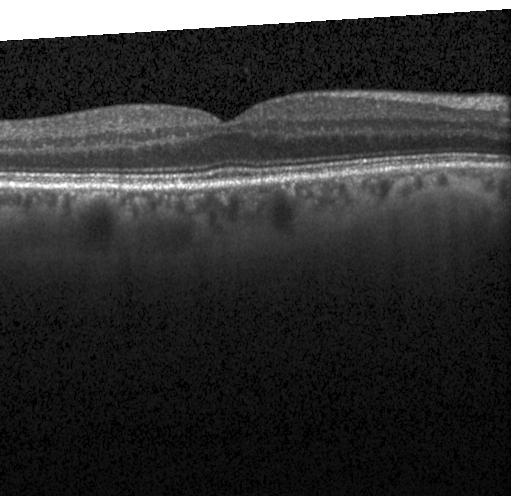
Centered on the fovea. Instrument: Heidelberg Spectralis. Retinal OCT B-scan. SD-OCT.
Diagnosis: no CNV, DME, or drusen.